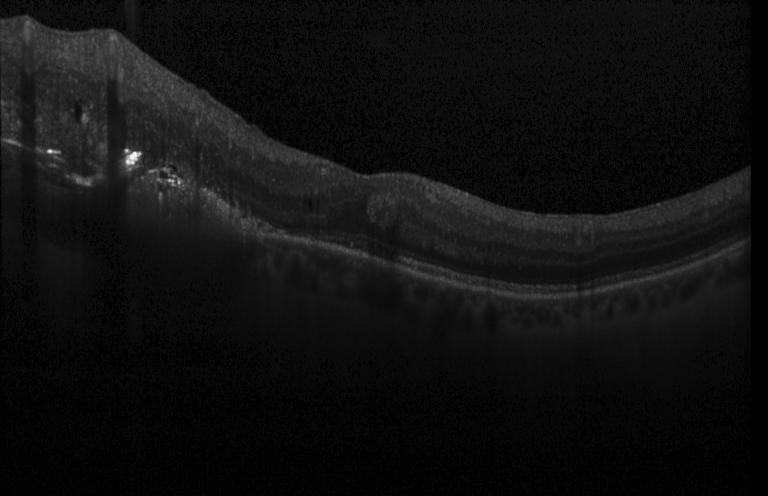

Macular OCT: choroidal neovascularization (CNV).